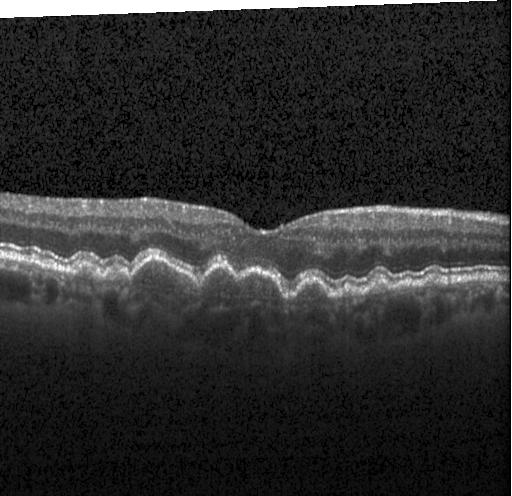

Sub-RPE drusenoid deposits.